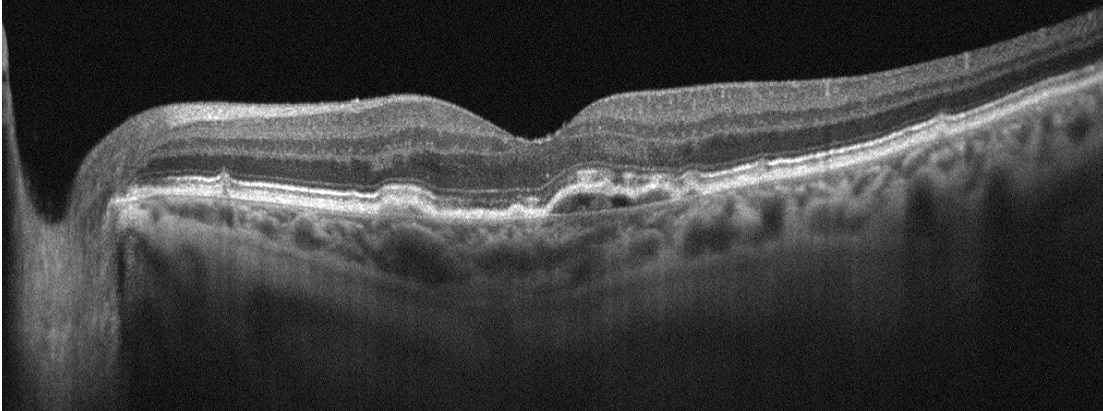
OCT finding: age-related macular degeneration (AMD).